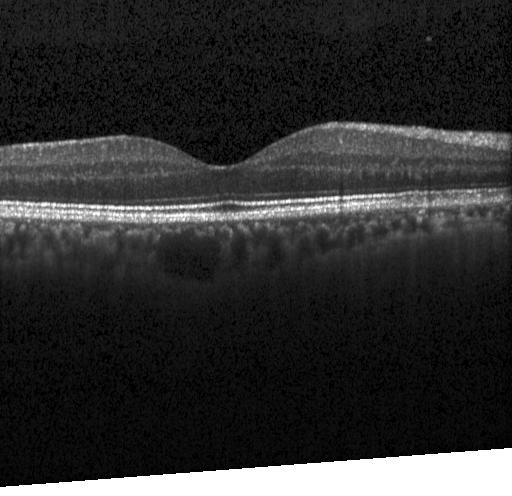
Impression: neither choroidal neovascularization, diabetic macular edema, nor drusen.